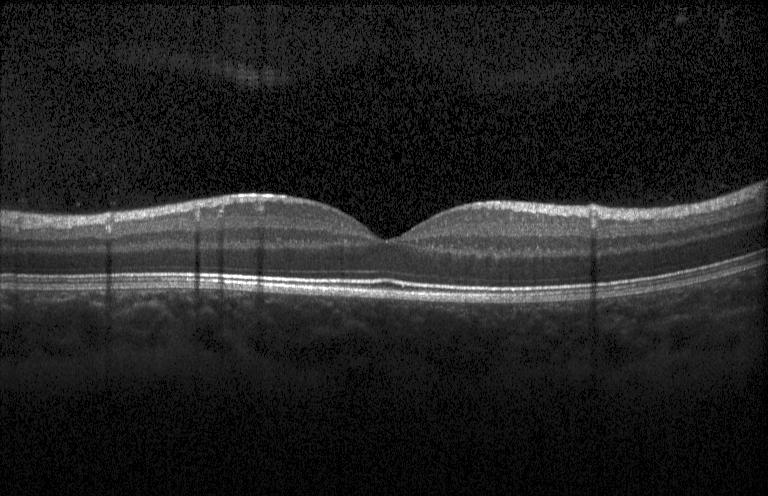
Optical coherence tomography B-scan; acquired on a Heidelberg Spectralis. Macular OCT: no choroidal neovascularization, no diabetic macular edema, and no drusen.